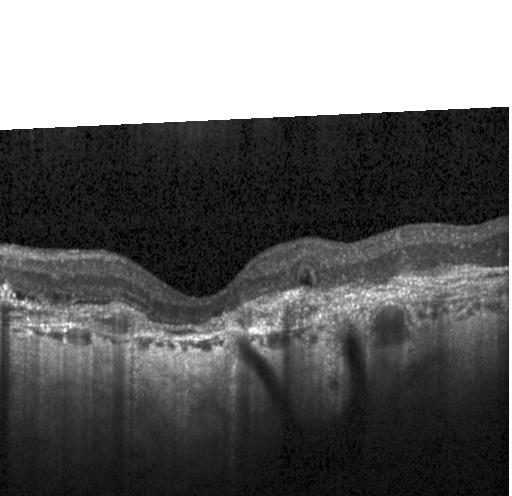
Acquired on a Heidelberg Spectralis · optical coherence tomography scan · spectral-domain OCT · horizontal scan through the fovea. Dx: CNV.